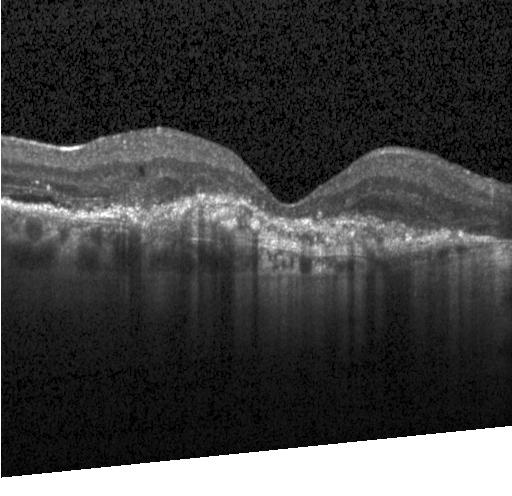
Macular scan. Retinal OCT cross-section
OCT finding: a choroidal neovascular membrane.